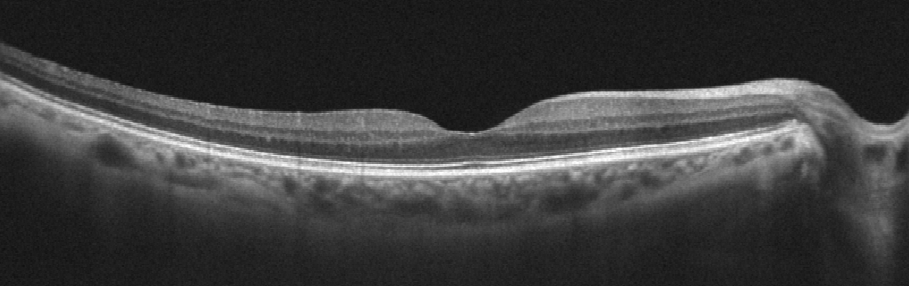
No AMD, DME, ERM, RAO, RVO, or VID.